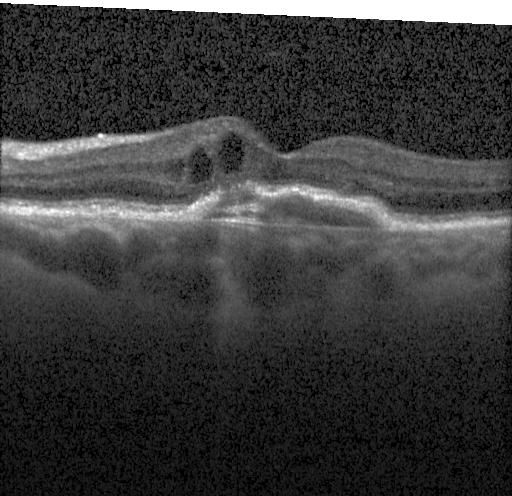 Acquired on a Heidelberg Spectralis, SD-OCT, OCT B-scan, fovea-centered.
Macular OCT: a choroidal neovascular membrane.